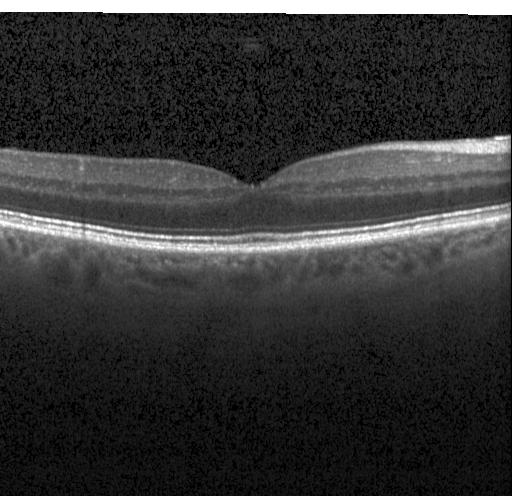 OCT scan showing neither CNV, DME, nor drusen.